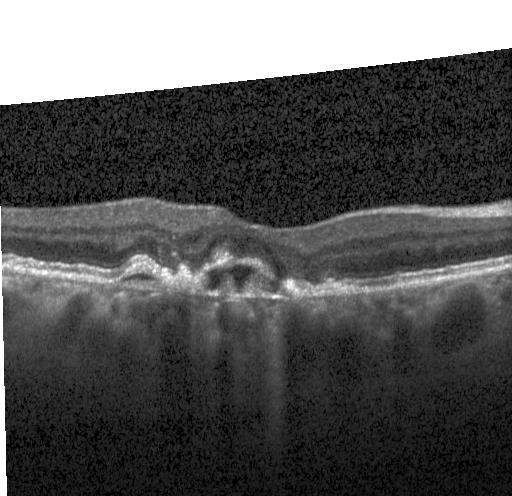

OCT line scan · fovea-centered · spectral-domain optical coherence tomography · Heidelberg Spectralis OCT system. Impression: a choroidal neovascular membrane.